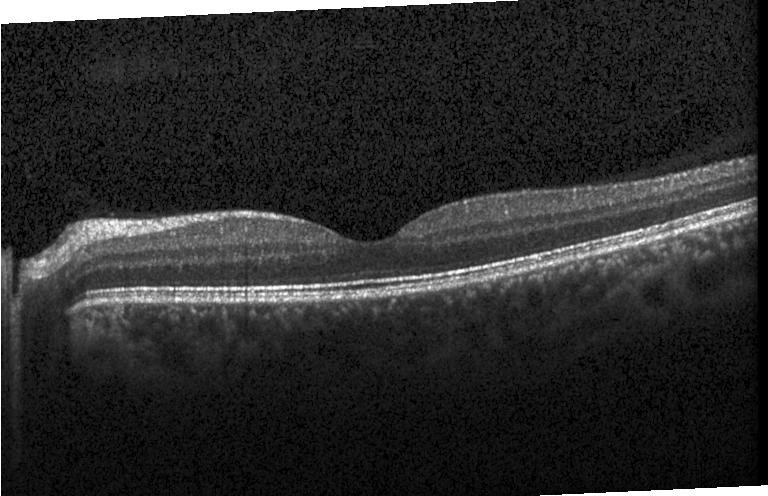

Optical coherence tomography B-scan — Assessment: no evidence of CNV, DME, or drusen.